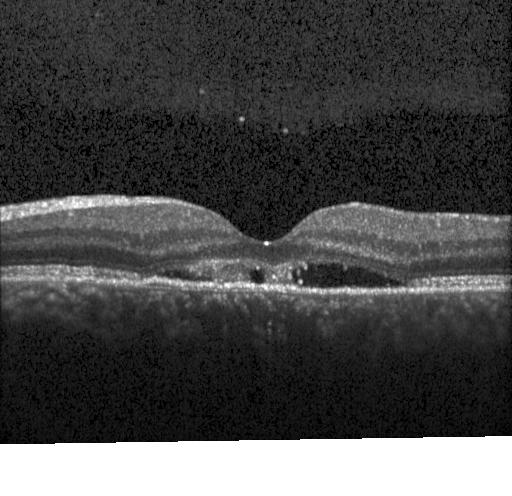

Macular OCT: a choroidal neovascular membrane.